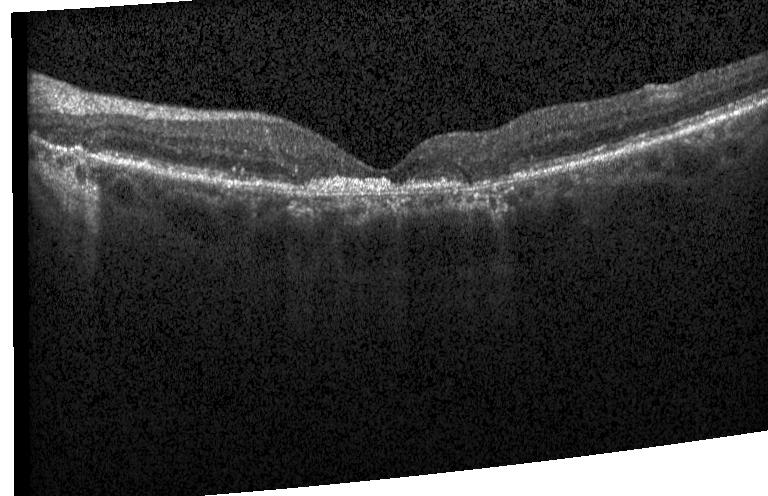 Horizontal scan through the fovea. Instrument: Heidelberg Spectralis. Retinal OCT B-scan
Diagnosis: a choroidal neovascular membrane.